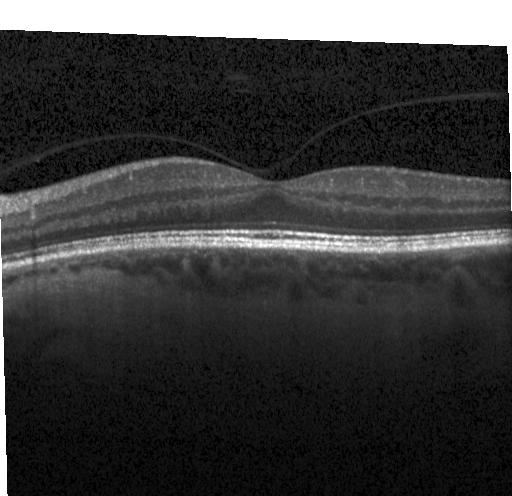

OCT finding: no choroidal neovascularization, diabetic macular edema, or drusen.